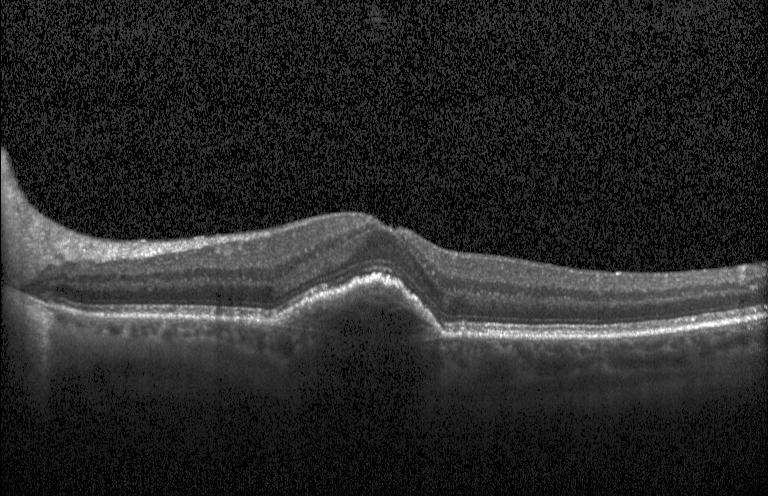
Finding: choroidal neovascularization (CNV).